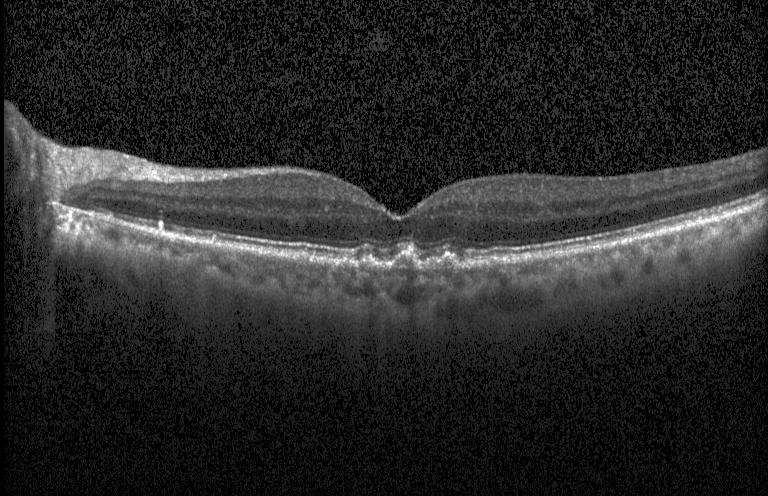 Centered on the fovea. Instrument: Heidelberg Spectralis. Retinal OCT cross-section. SD-OCT.
Impression: sub-RPE drusenoid deposits.